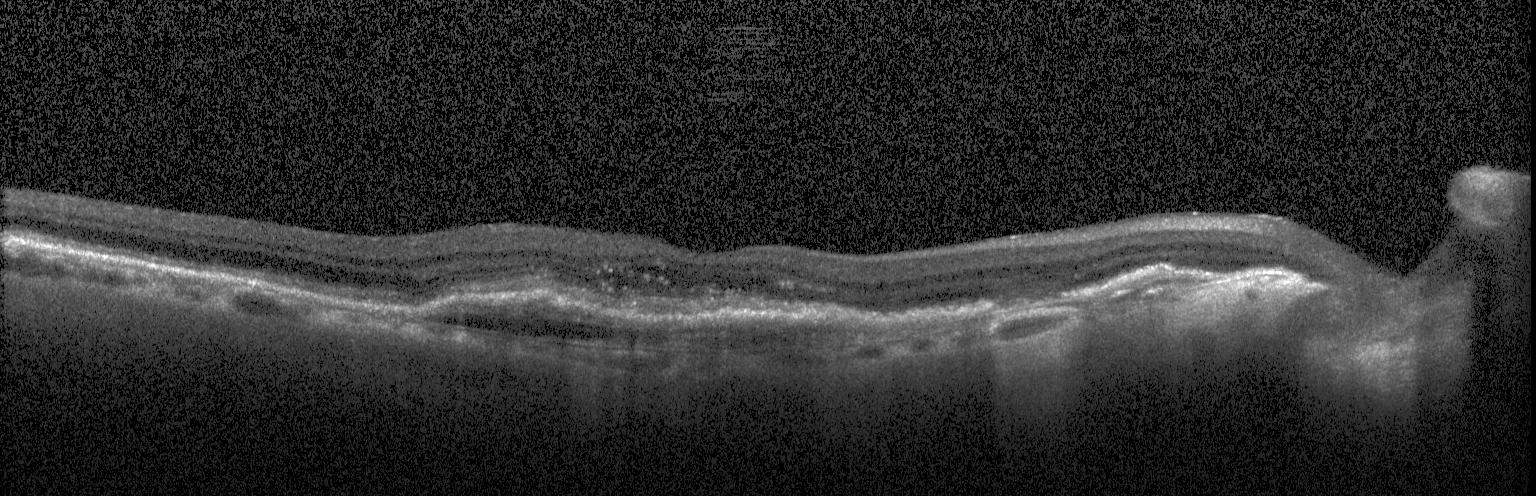 OCT finding: a choroidal neovascular membrane.